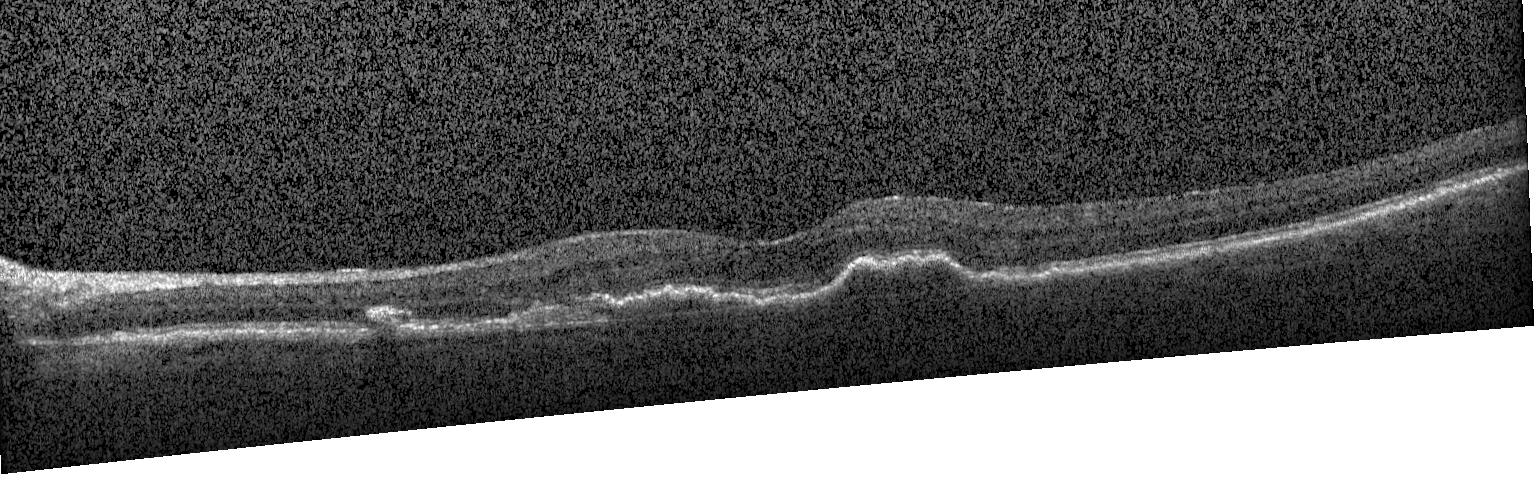 OCT line scan. Dx: choroidal neovascularization.